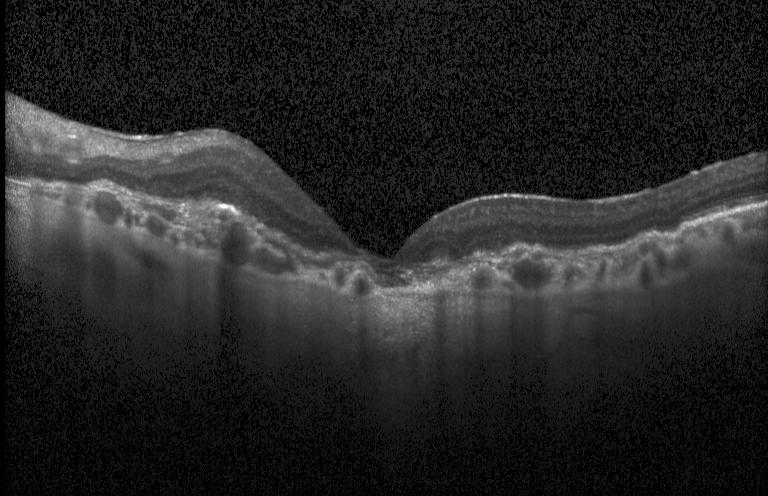 OCT line scan · Heidelberg Spectralis OCT system — This B-scan demonstrates a choroidal neovascular membrane.